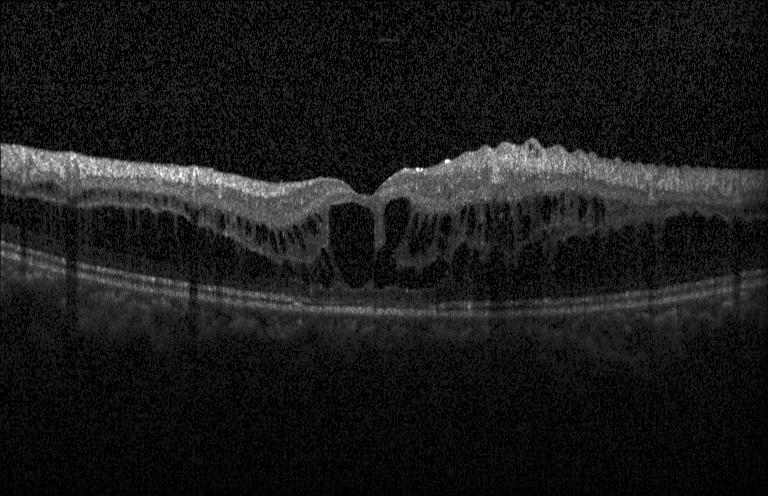 Retinal OCT B-scan; spectral-domain OCT; centered on the fovea.
OCT finding: diabetic macular edema.